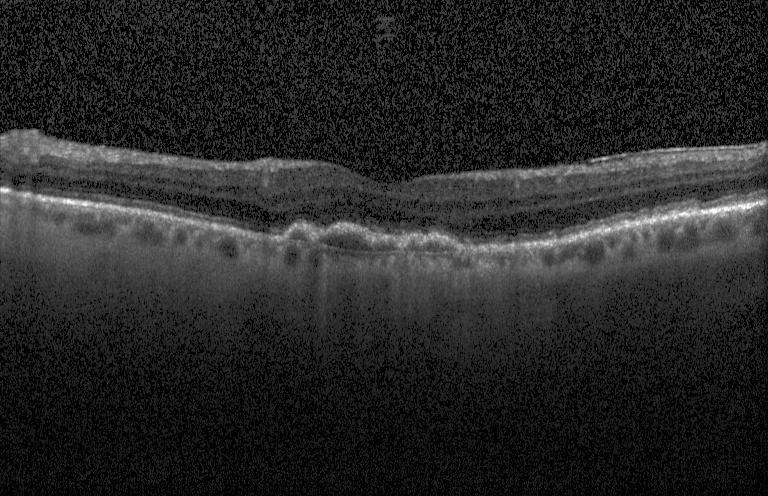

SD-OCT; optical coherence tomography B-scan
Assessment: choroidal neovascularization.